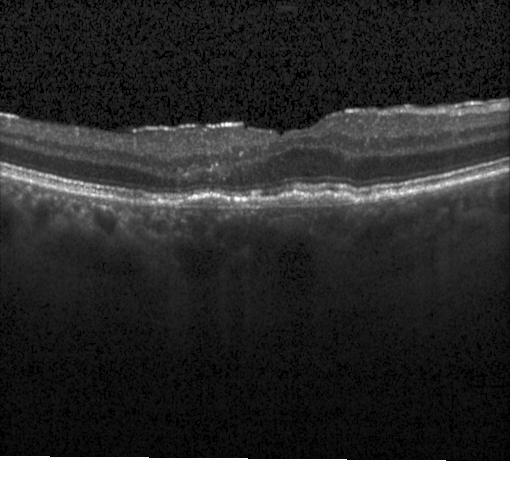

Spectral-domain OCT · OCT B-scan · through the macula · instrument: Heidelberg Spectralis — Impression: choroidal neovascularization (CNV).